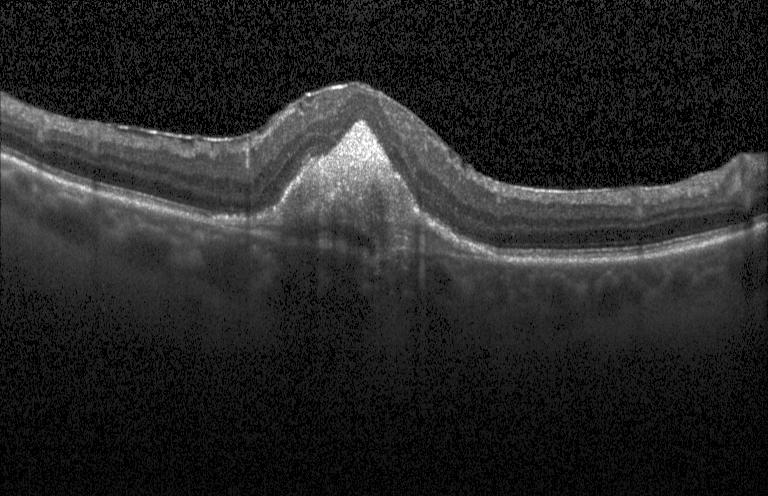 Assessment: a choroidal neovascular membrane.